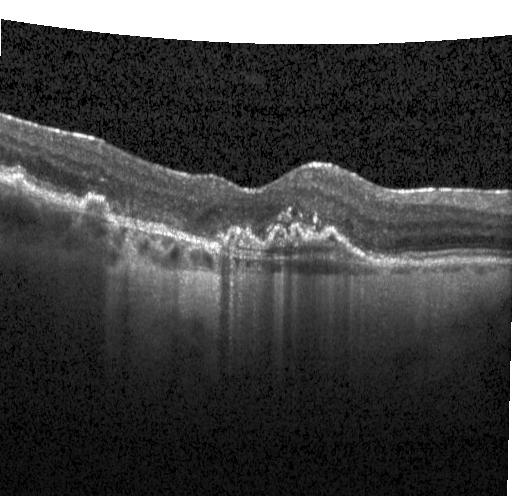

OCT finding: a choroidal neovascular membrane.